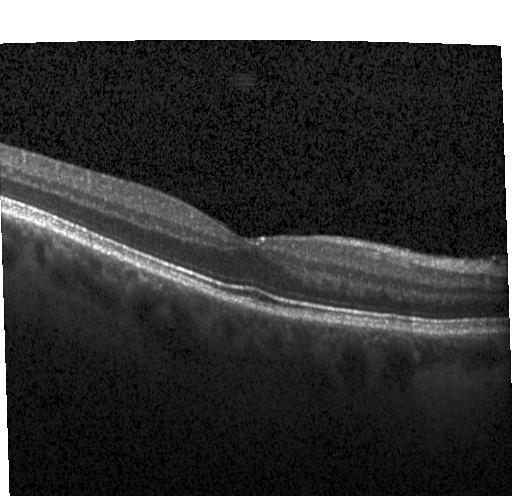
Horizontal scan through the fovea · OCT B-scan
The scan shows no CNV, no DME, and no drusen.